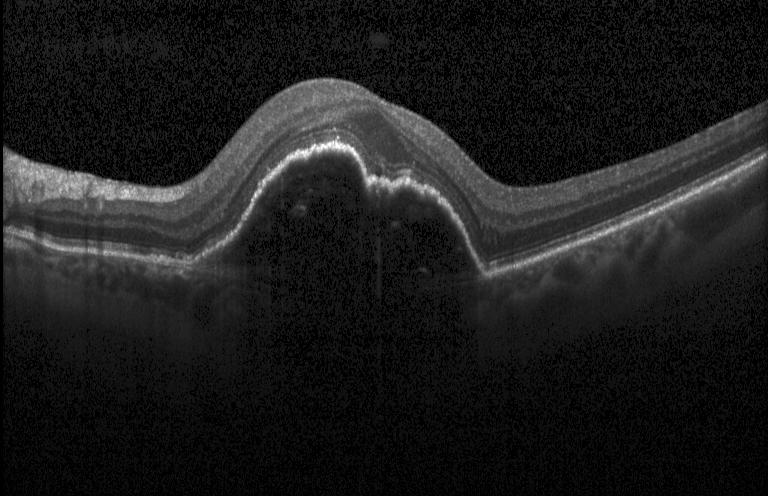 Spectral-domain OCT, optical coherence tomography B-scan.
Finding: CNV.